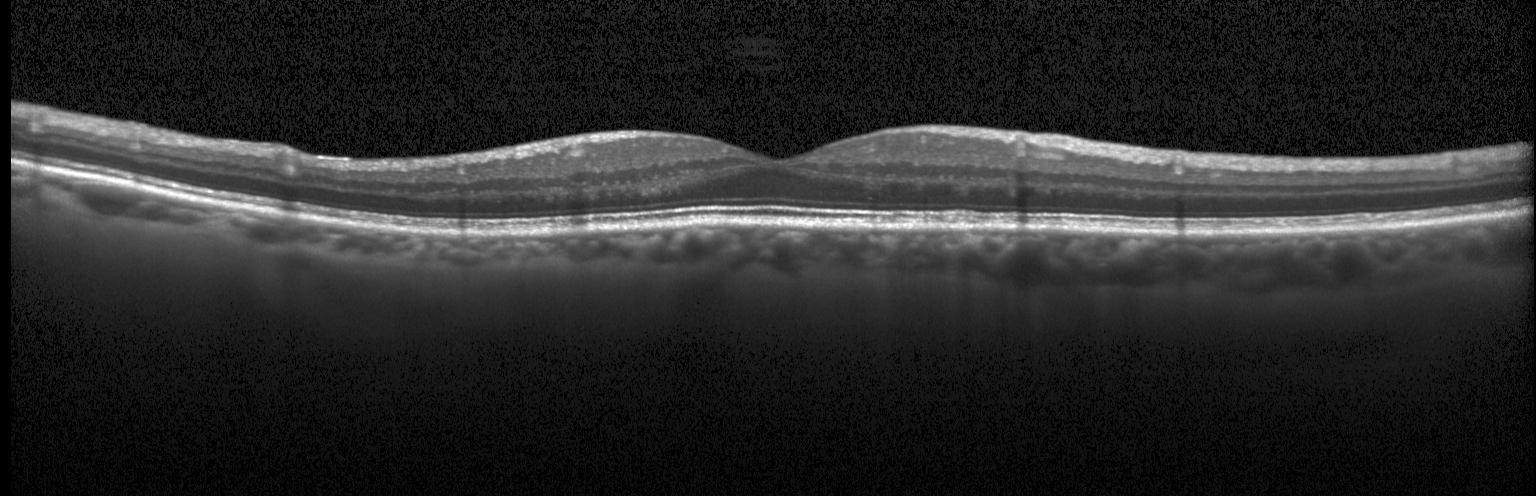

OCT B-scan · horizontal scan through the fovea.
Impression: neither choroidal neovascularization, diabetic macular edema, nor drusen.